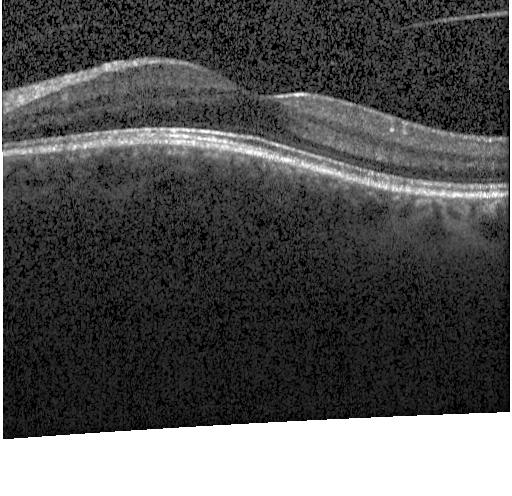

The scan shows no choroidal neovascularization, no diabetic macular edema, and no drusen.